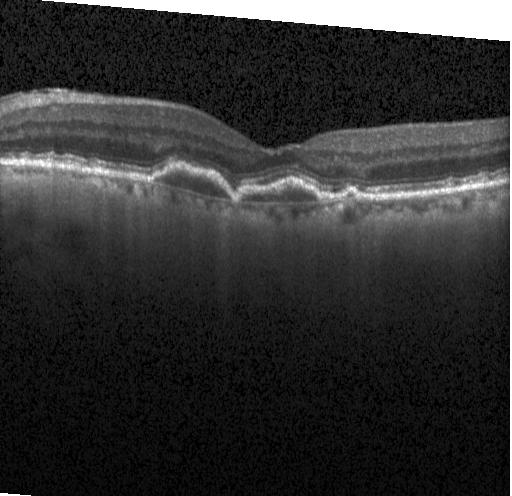
Heidelberg Spectralis; optical coherence tomography scan; fovea-centered; SD-OCT — Dx: a choroidal neovascular membrane.